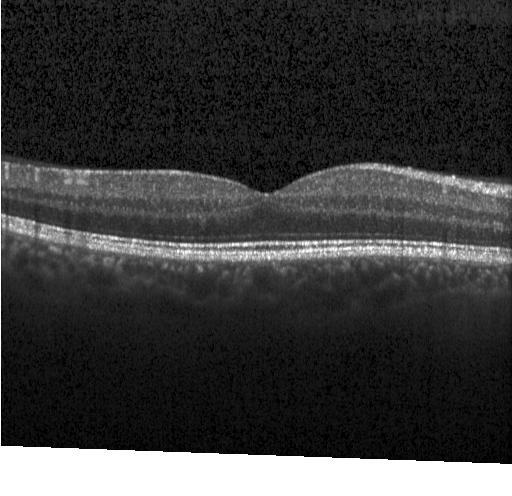
OCT B-scan showing no CNV, no DME, and no drusen.